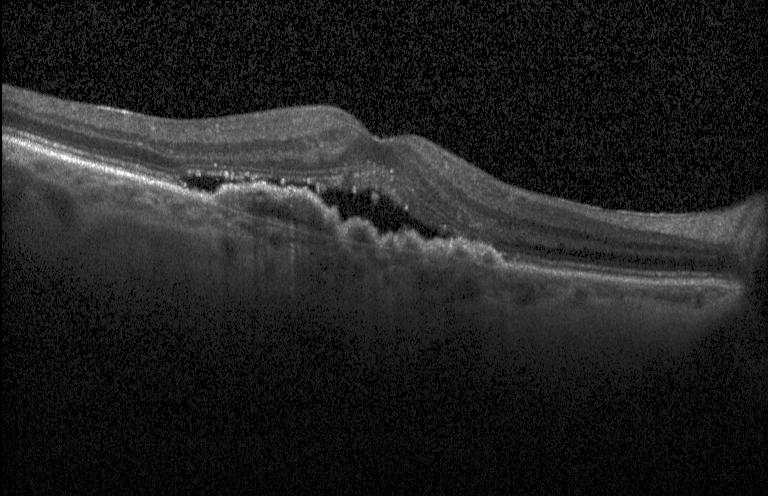 OCT line scan · acquired on a Heidelberg Spectralis · horizontal scan through the fovea. Macular OCT: a choroidal neovascular membrane.